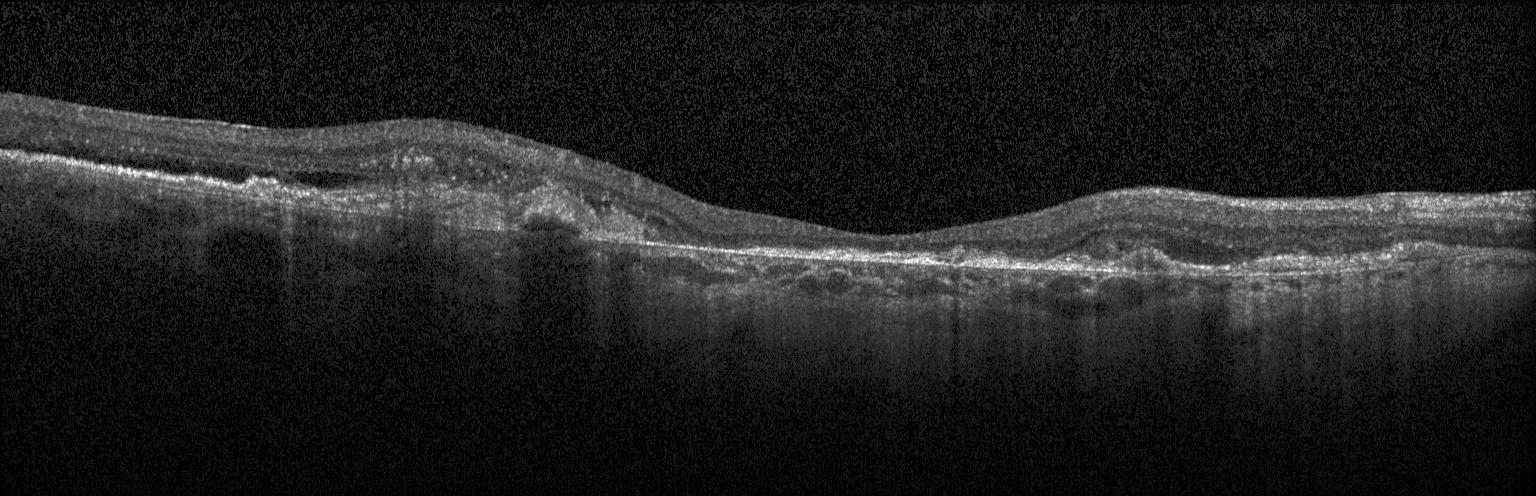
Retinal OCT cross-section showing a choroidal neovascular membrane.